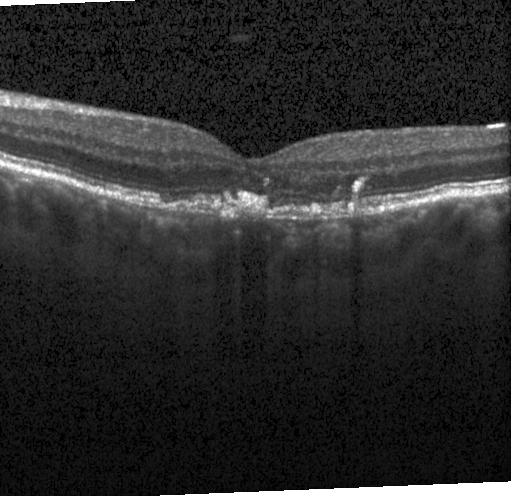
Spectral-domain optical coherence tomography, acquired on a Heidelberg Spectralis, OCT line scan, centered on the fovea.
This B-scan demonstrates choroidal neovascularization.